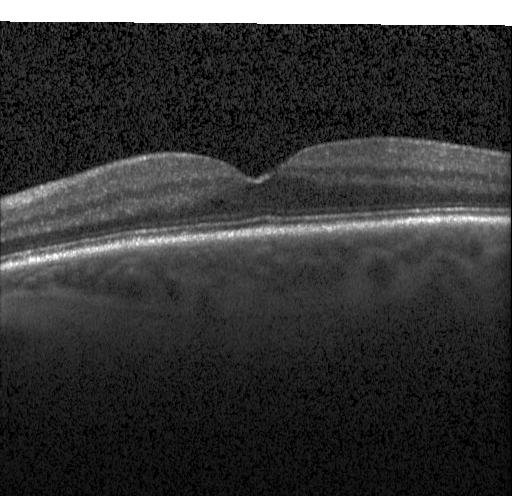
Assessment: neither CNV, DME, nor drusen.